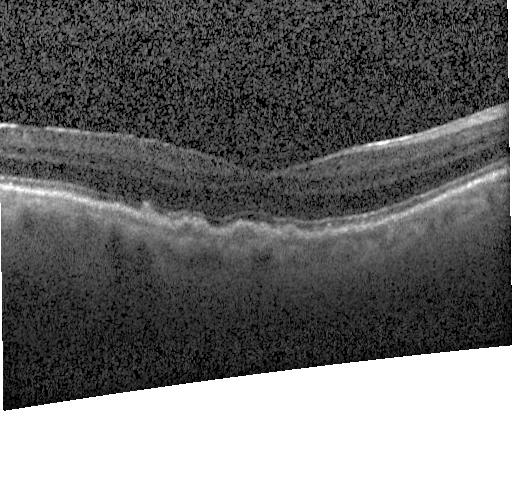
OCT finding: choroidal neovascularization (CNV).